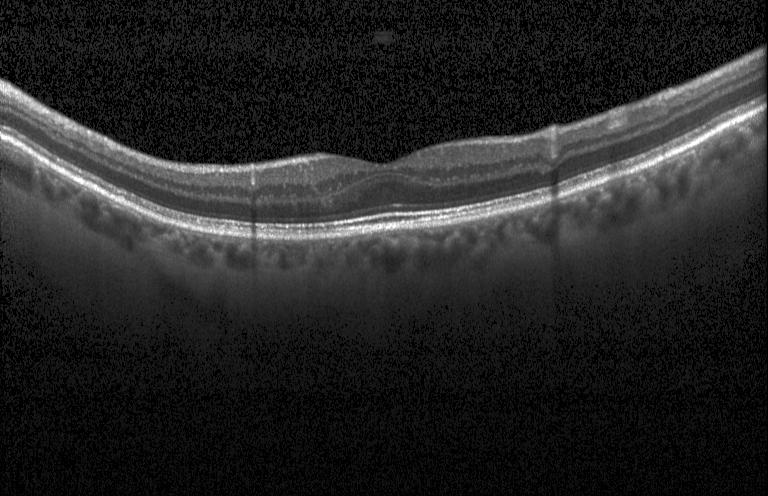
Optical coherence tomography B-scan.
Diagnosis: no choroidal neovascularization, no diabetic macular edema, and no drusen.